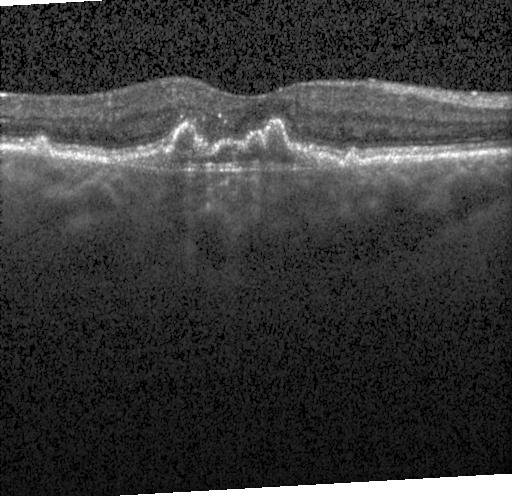
OCT B-scan · acquired on a Heidelberg Spectralis.
Assessment: CNV.